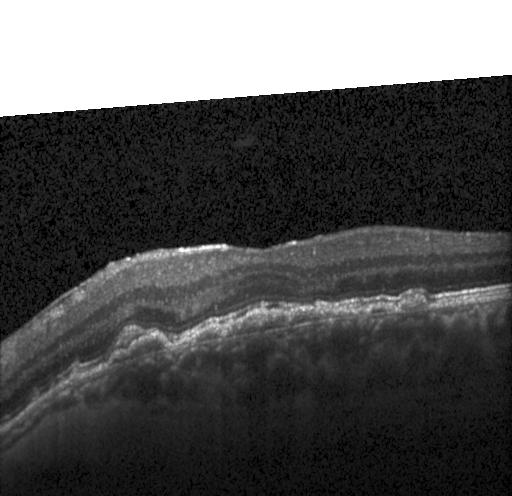

Fovea-centered; retinal OCT B-scan; spectral-domain optical coherence tomography — Macular OCT: a choroidal neovascular membrane.